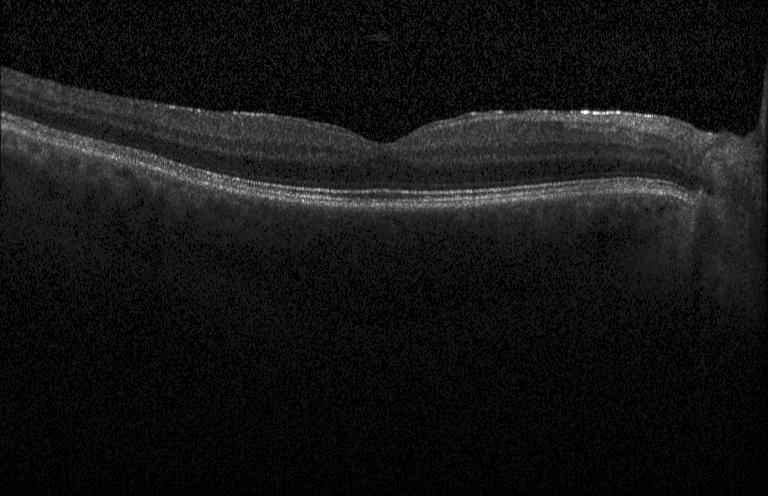
OCT finding: no choroidal neovascularization, diabetic macular edema, or drusen.